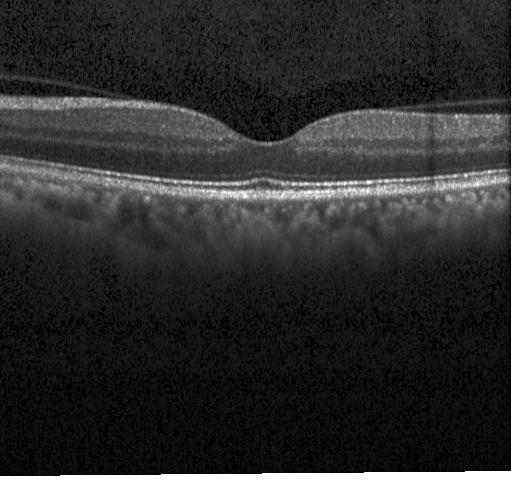

Optical coherence tomography B-scan · horizontal scan through the fovea. The scan shows neither choroidal neovascularization, diabetic macular edema, nor drusen.